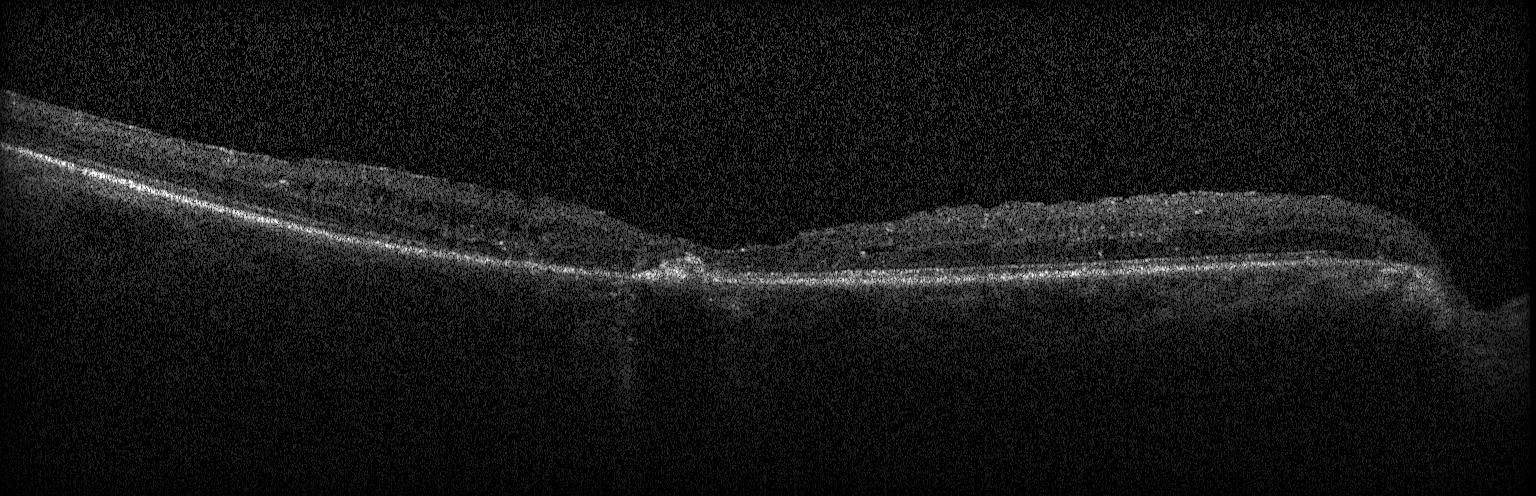
Finding: CNV.